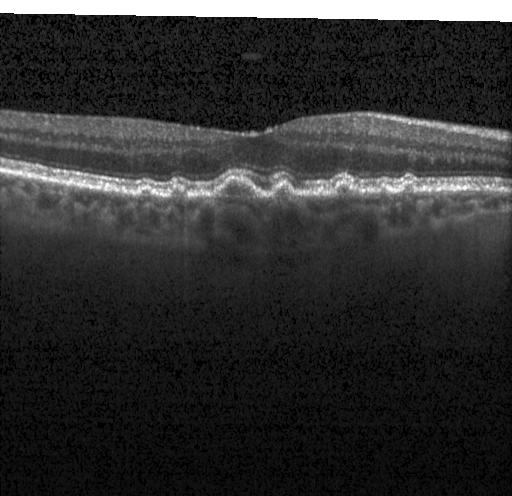 OCT B-scan showing drusen.